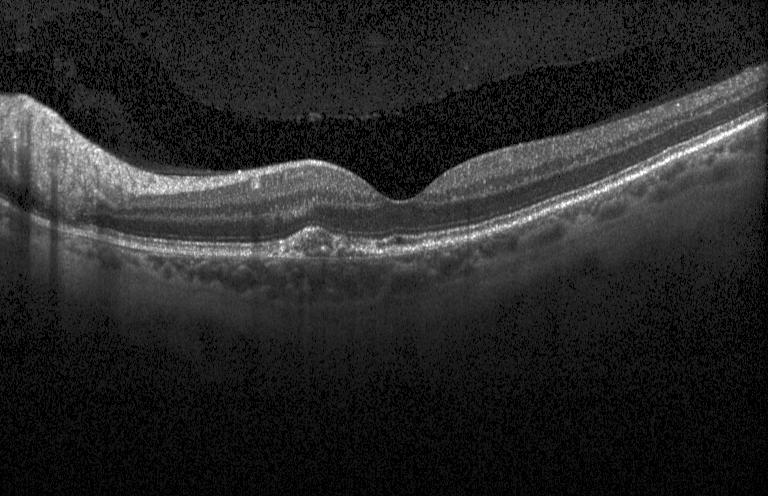 OCT line scan.
Choroidal neovascularization (CNV).